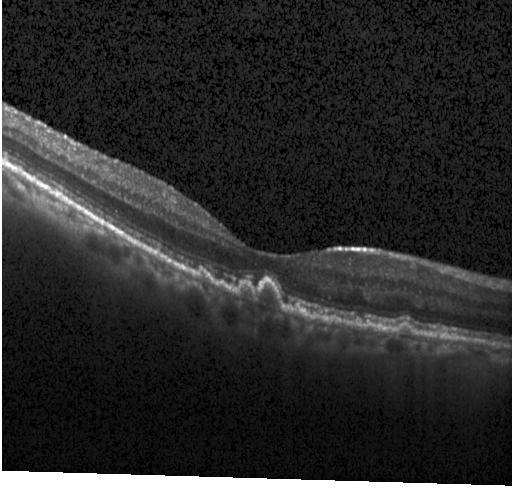

Spectral-domain OCT B-scan: multiple drusen.